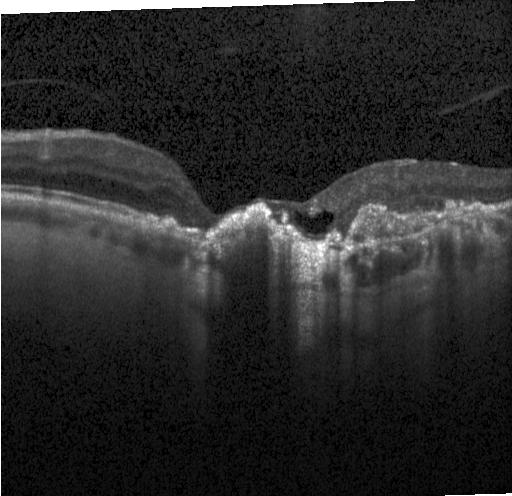 Acquired on a Heidelberg Spectralis; OCT line scan; SD-OCT; through the macula
Diagnosis: CNV.